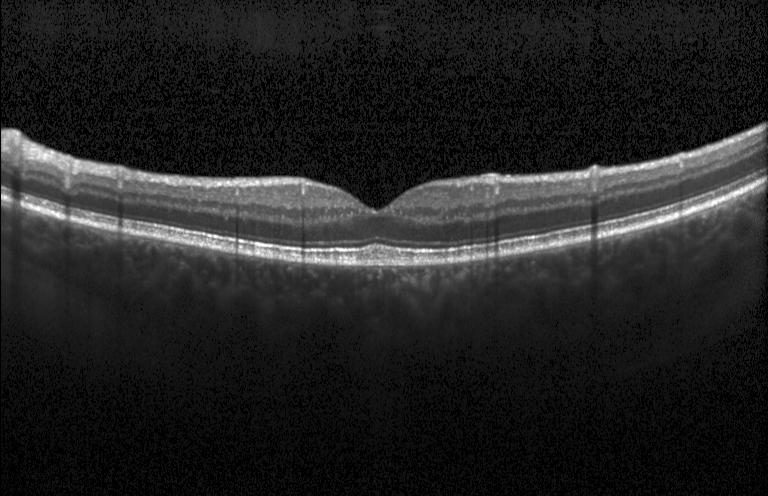
Acquired on a Heidelberg Spectralis, SD-OCT, through the macula, OCT line scan
Finding: no choroidal neovascularization, no diabetic macular edema, and no drusen.